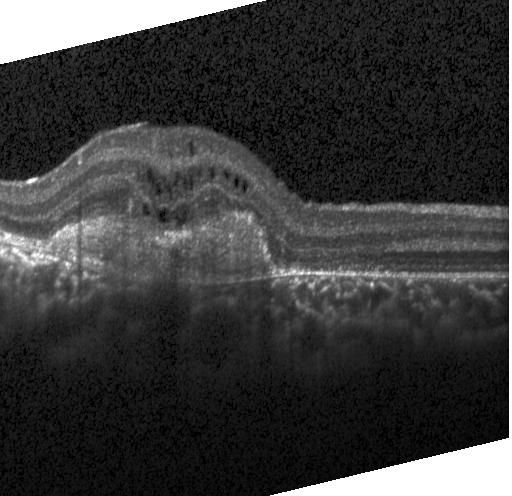
Spectral-domain optical coherence tomography · OCT line scan — Impression: choroidal neovascularization (CNV).